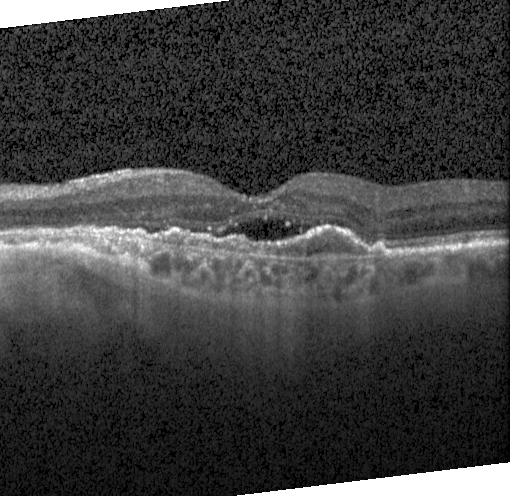

Macular scan · SD-OCT · optical coherence tomography B-scan
OCT finding: choroidal neovascularization (CNV).